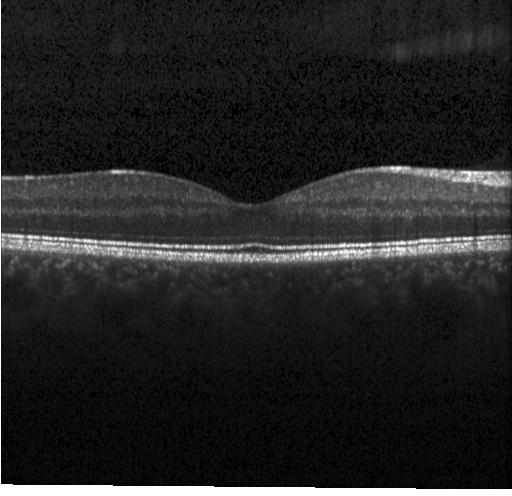 Optical coherence tomography scan
This B-scan demonstrates no choroidal neovascularization, diabetic macular edema, or drusen.